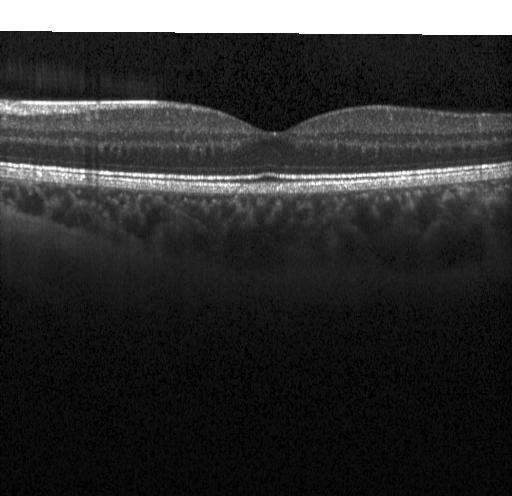 Retinal OCT B-scan. Diagnosis: no evidence of choroidal neovascularization, diabetic macular edema, or drusen.